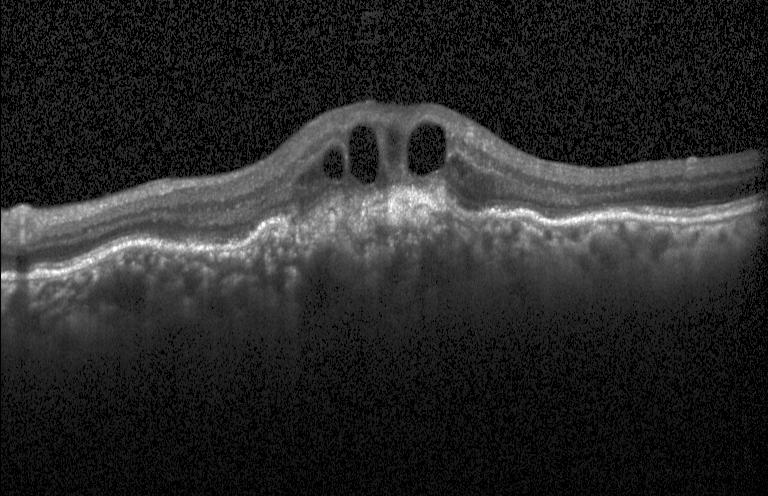
OCT line scan; acquired on a Heidelberg Spectralis. OCT finding: a choroidal neovascular membrane.